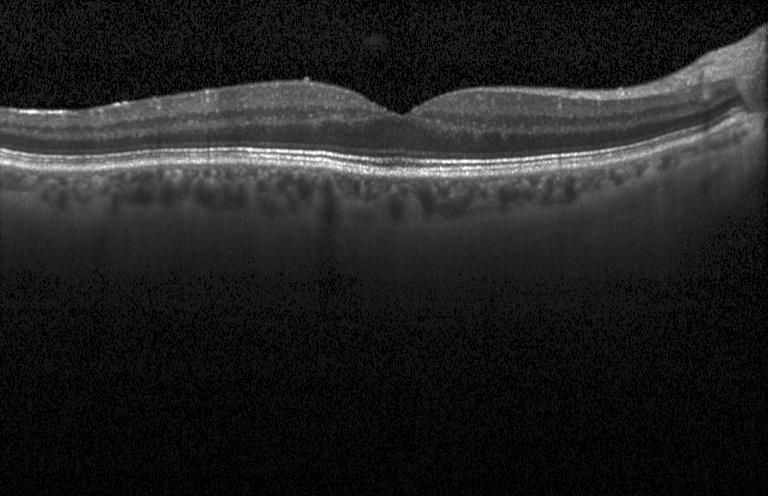
Spectral-domain OCT. Optical coherence tomography B-scan
Finding: no CNV, no DME, and no drusen.